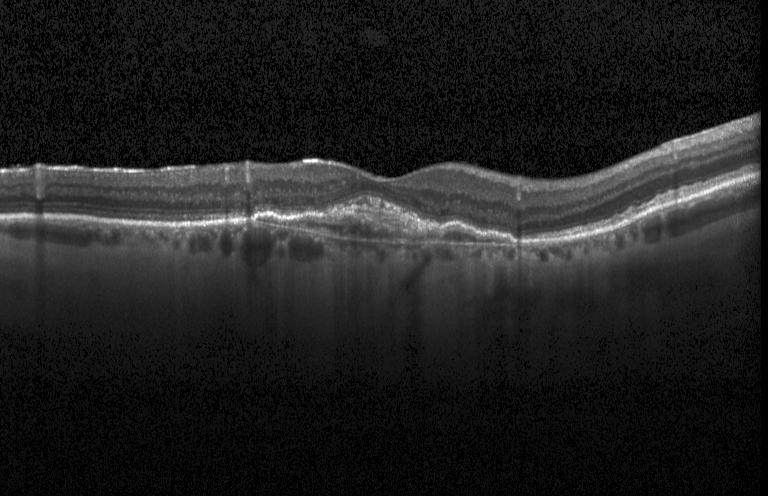

OCT B-scan showing a choroidal neovascular membrane.